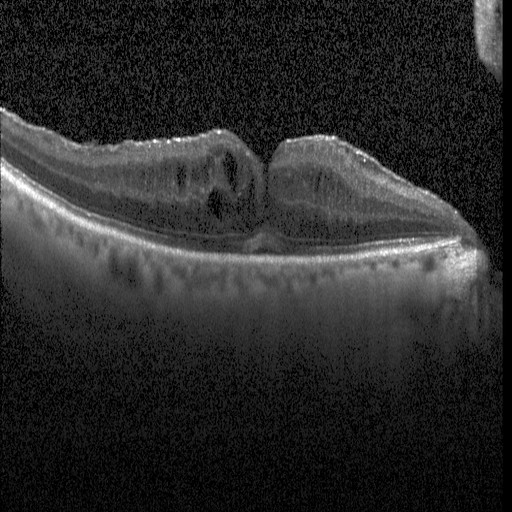
Finding: diabetic macular edema (DME).